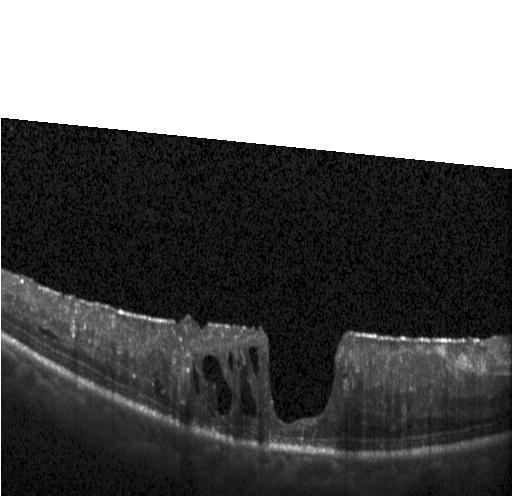 OCT B-scan, through the macula, instrument: Heidelberg Spectralis
Diabetic macular edema.